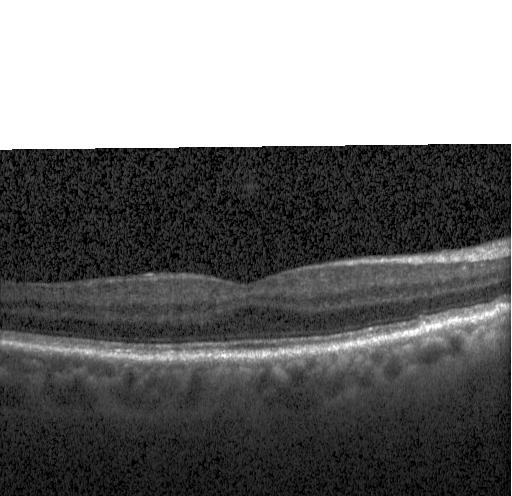 Horizontal scan through the fovea, Heidelberg Spectralis, OCT B-scan — Neither CNV, DME, nor drusen.